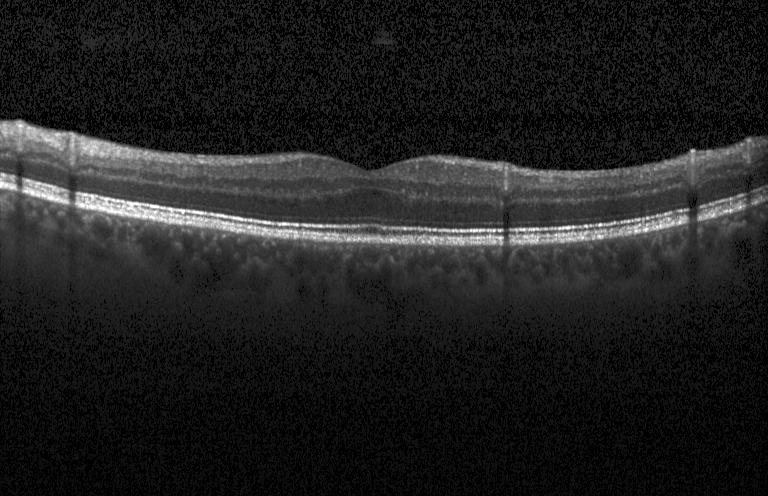 Retinal OCT cross-section
Diagnosis: no CNV, DME, or drusen.